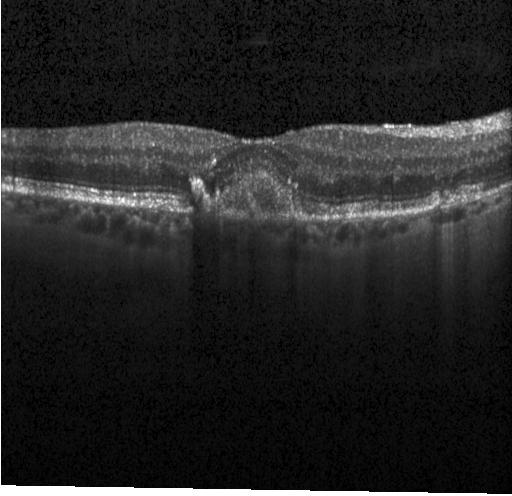
The scan shows a choroidal neovascular membrane.